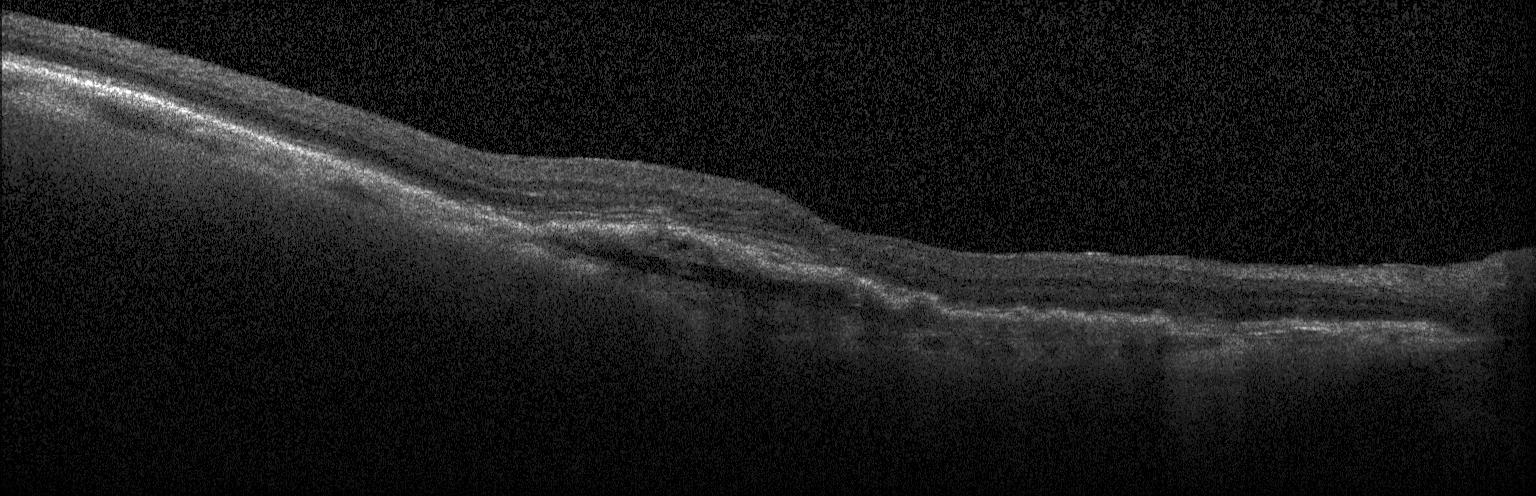

Finding: a choroidal neovascular membrane.